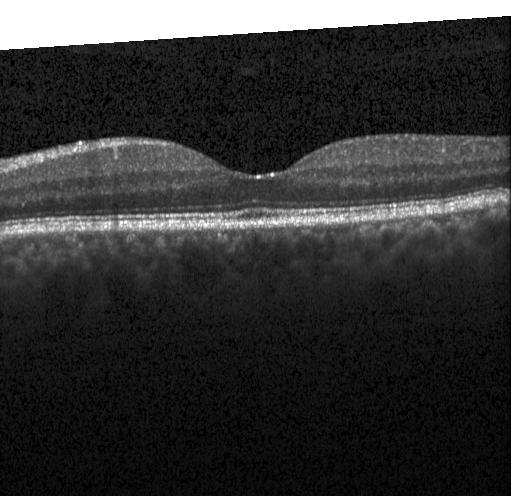

Centered on the fovea · retinal OCT cross-section · instrument: Heidelberg Spectralis · spectral-domain OCT
Impression: no choroidal neovascularization, diabetic macular edema, or drusen.